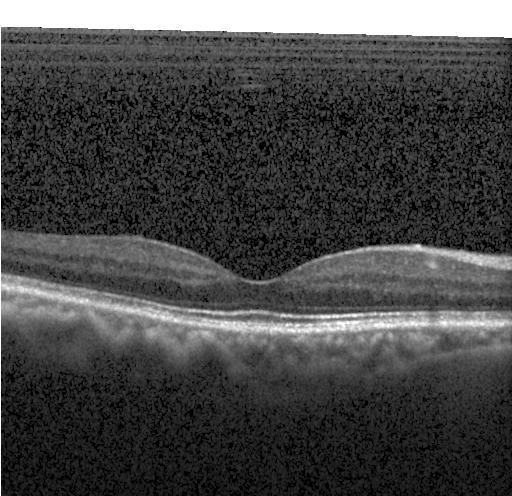
Retinal OCT B-scan
Impression: no choroidal neovascularization, diabetic macular edema, or drusen.